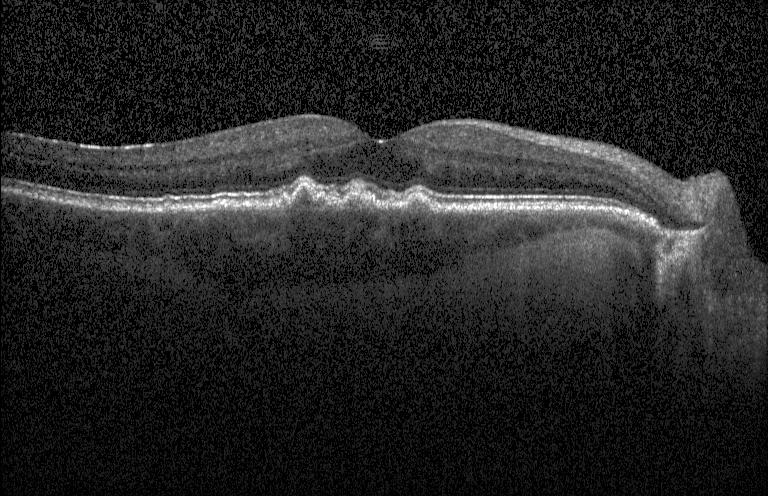 Diagnosis: multiple drusen.